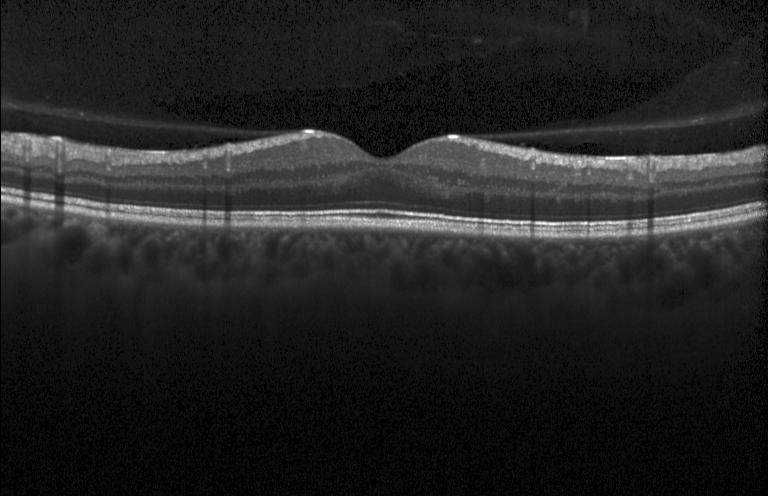
Retinal OCT cross-section showing no choroidal neovascularization, diabetic macular edema, or drusen.